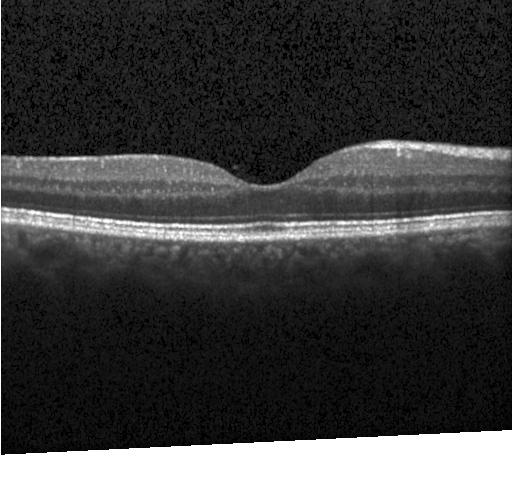 Assessment: no evidence of choroidal neovascularization, diabetic macular edema, or drusen.